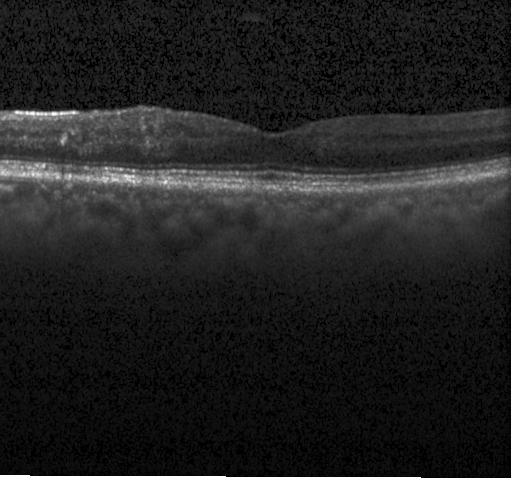
OCT line scan; Heidelberg Spectralis OCT system.
Diagnosis: neither CNV, DME, nor drusen.